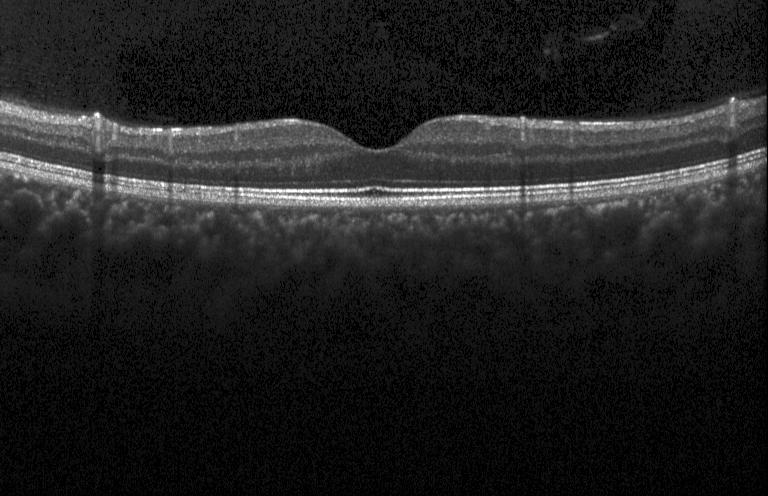

OCT line scan · spectral-domain OCT · instrument: Heidelberg Spectralis — Assessment: no CNV, DME, or drusen.